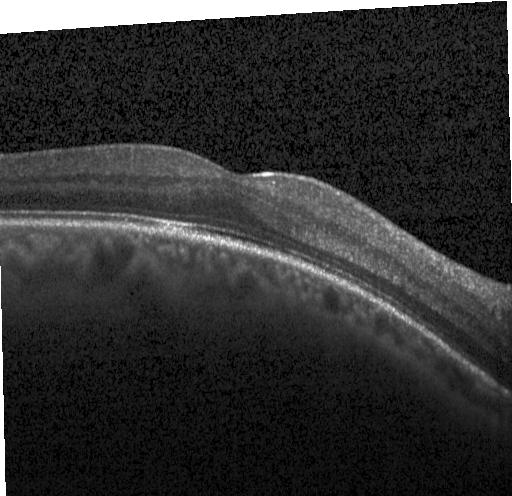 Assessment: no evidence of CNV, DME, or drusen.